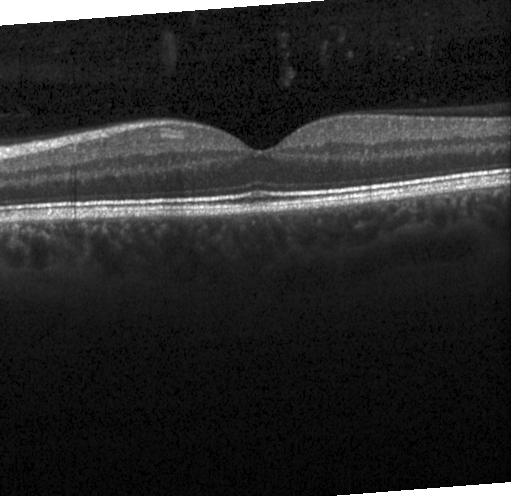

Heidelberg Spectralis · OCT line scan · through the macula — No evidence of CNV, DME, or drusen.